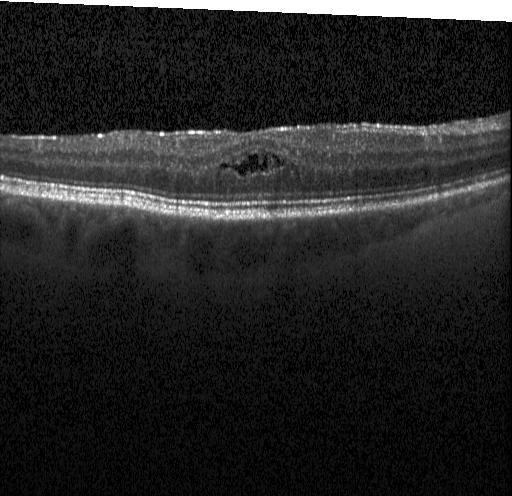

Spectral-domain OCT B-scan: diabetic macular edema.